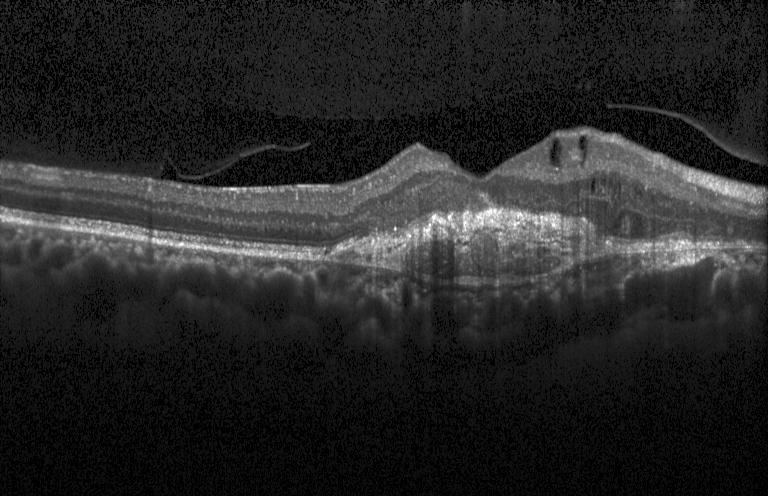

Heidelberg Spectralis OCT system. OCT line scan. Macular scan. Impression: a choroidal neovascular membrane.